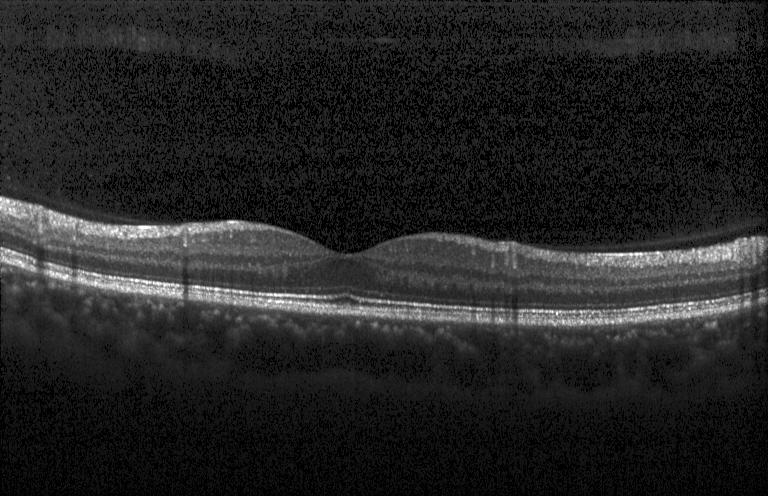 Optical coherence tomography scan · acquired on a Heidelberg Spectralis
Impression: no choroidal neovascularization, diabetic macular edema, or drusen.